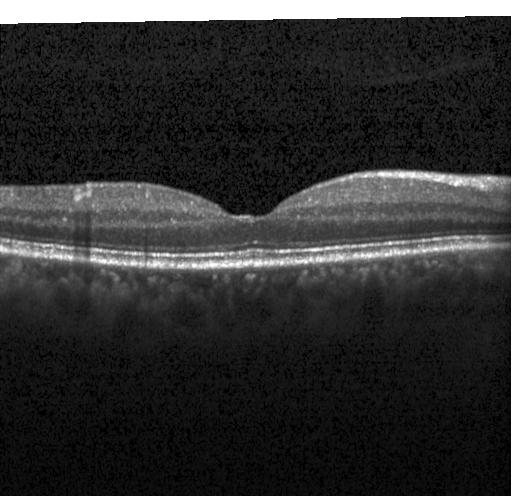

SD-OCT. Acquired on a Heidelberg Spectralis. Retinal OCT B-scan. Through the macula. Finding: neither choroidal neovascularization, diabetic macular edema, nor drusen.